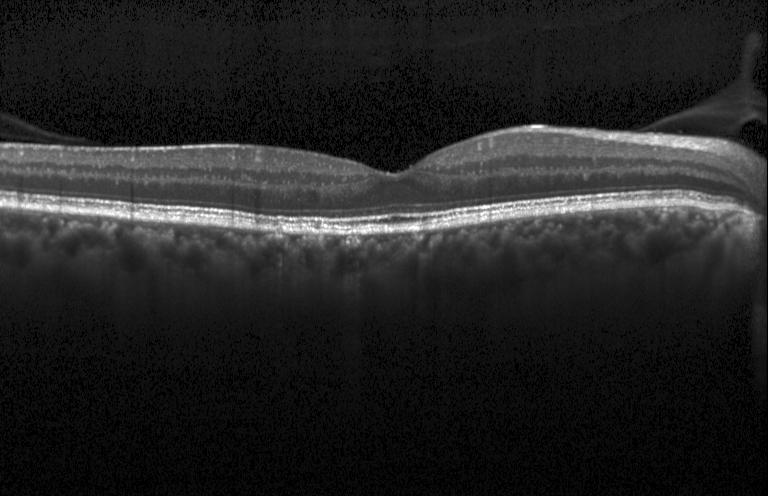 Fovea-centered, OCT B-scan — No choroidal neovascularization, diabetic macular edema, or drusen.